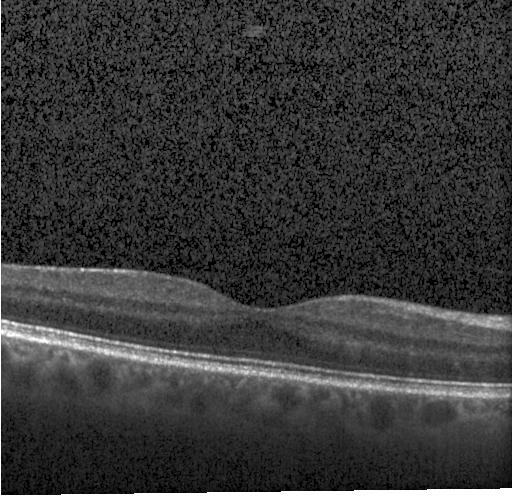

Spectral-domain OCT, through the macula, retinal OCT B-scan — Diagnosis: neither CNV, DME, nor drusen.